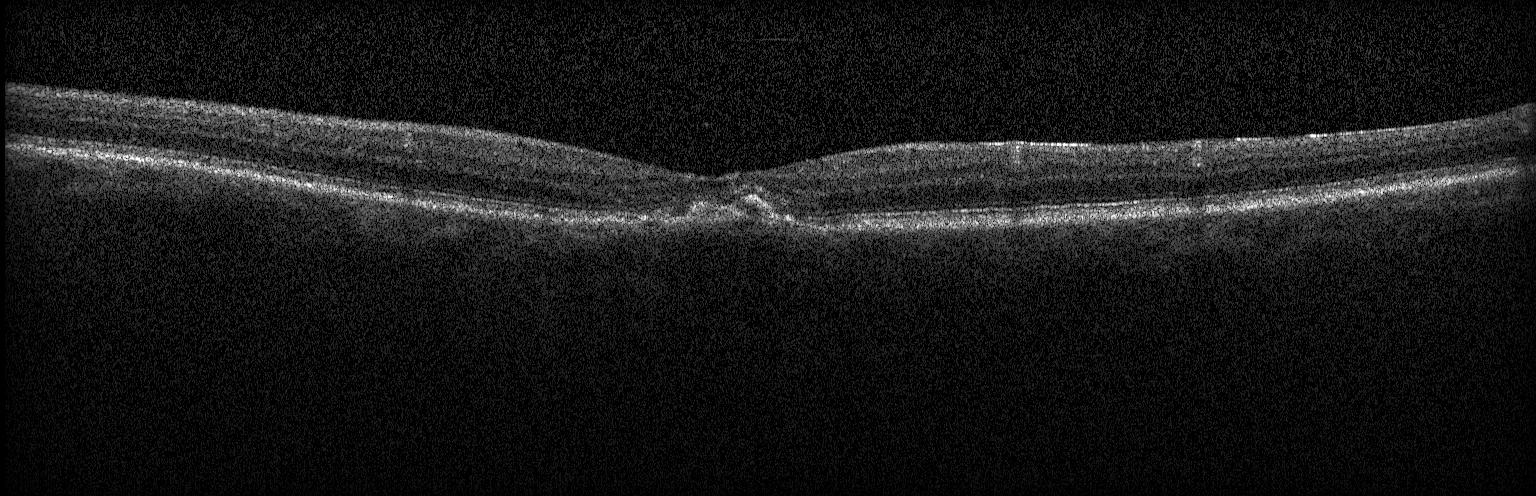
OCT line scan. Instrument: Heidelberg Spectralis. Spectral-domain OCT. Centered on the fovea — The scan shows CNV.